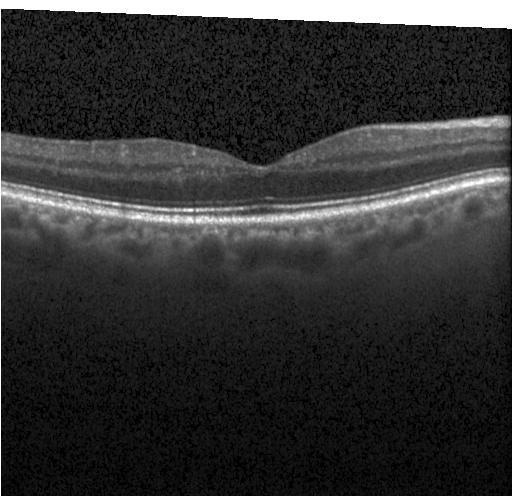
Centered on the fovea. Instrument: Heidelberg Spectralis. Optical coherence tomography scan.
Neither choroidal neovascularization, diabetic macular edema, nor drusen.